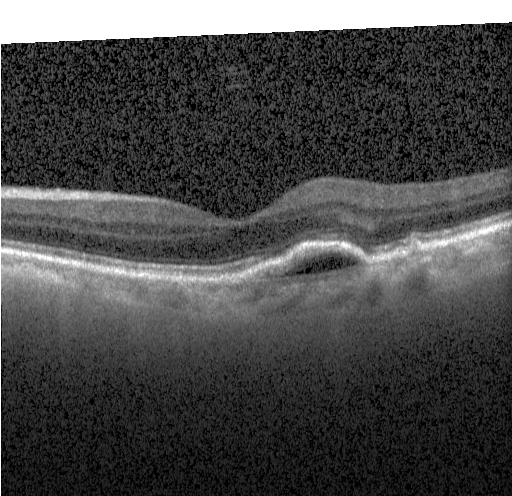

Instrument: Heidelberg Spectralis · centered on the fovea · retinal OCT cross-section.
Finding: choroidal neovascularization.